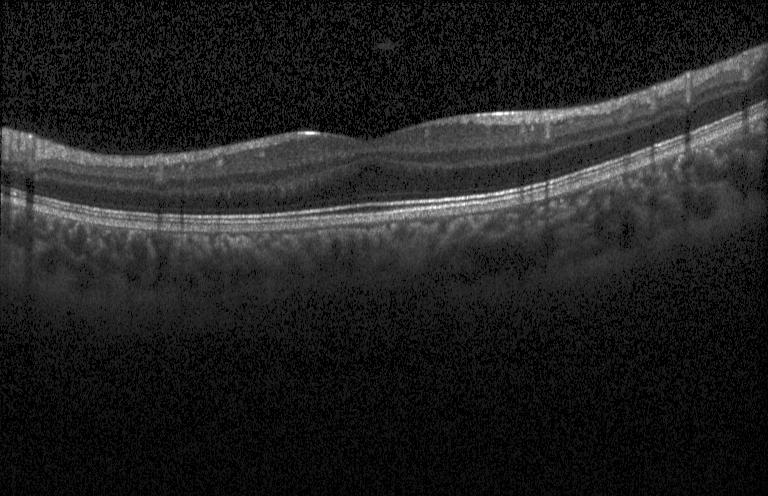
Retinal OCT cross-section. Spectral-domain OCT. Through the macula.
Diagnosis: no CNV, DME, or drusen.